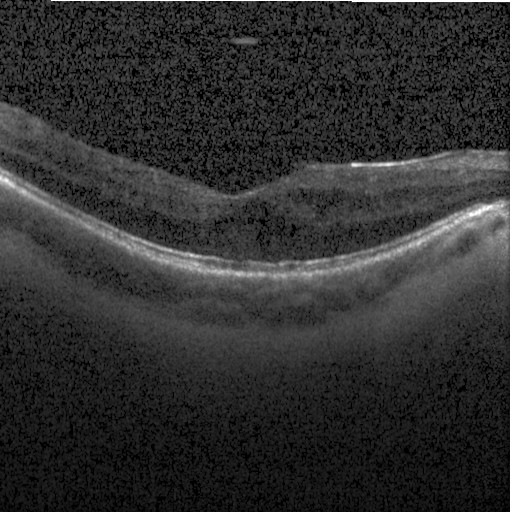

Retinal OCT cross-section showing diabetic macular edema.